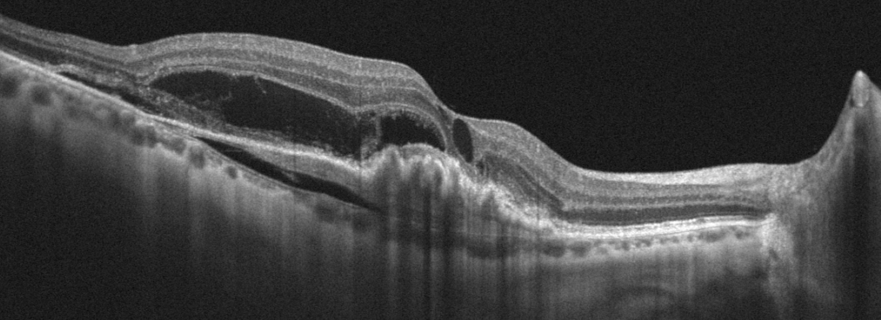

OCT line scan. Macular scan — Diagnosis: age-related macular degeneration.